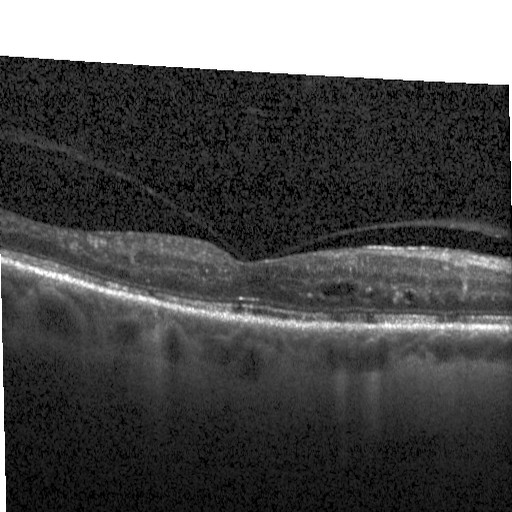
Heidelberg Spectralis OCT system; macular scan; retinal OCT cross-section; spectral-domain OCT.
Impression: diabetic macular edema (DME).